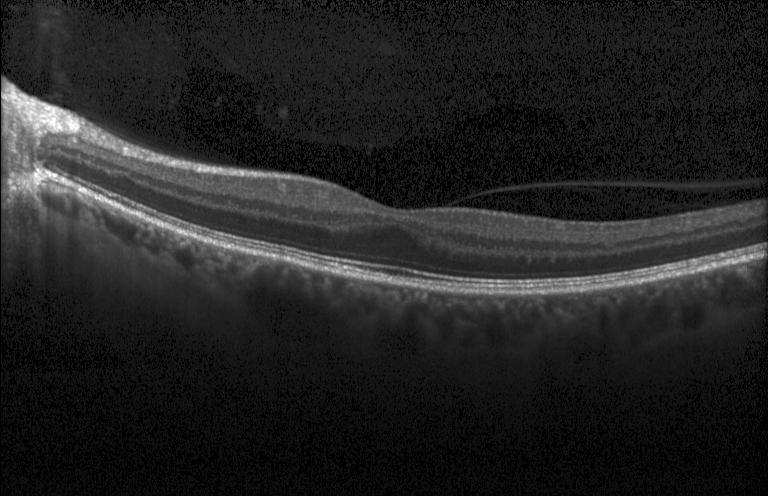
SD-OCT, OCT B-scan.
This B-scan demonstrates neither choroidal neovascularization, diabetic macular edema, nor drusen.